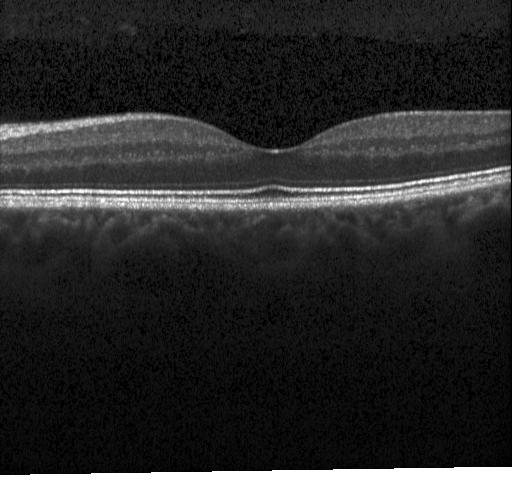
OCT B-scan · horizontal scan through the fovea · instrument: Heidelberg Spectralis — Macular OCT: neither CNV, DME, nor drusen.